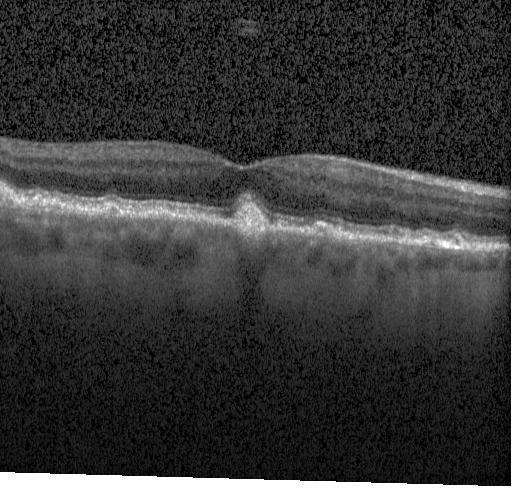

Horizontal scan through the fovea. Acquired on a Heidelberg Spectralis. Optical coherence tomography B-scan
Impression: drusen.